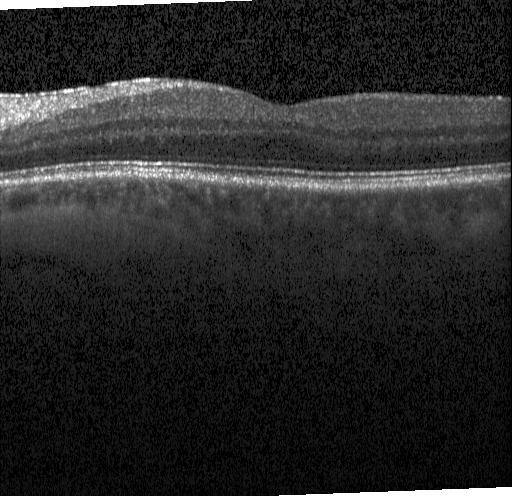
Retinal OCT cross-section — Finding: neither CNV, DME, nor drusen.